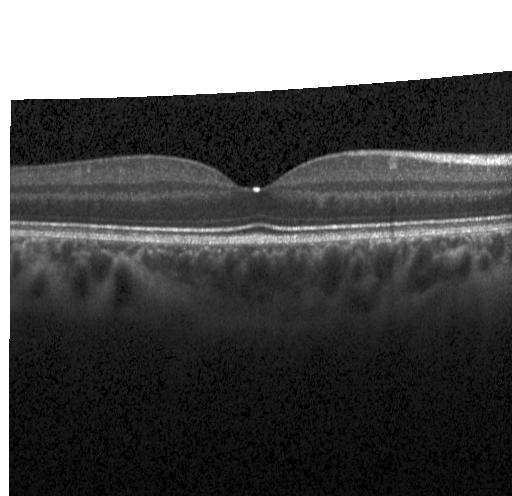

SD-OCT, instrument: Heidelberg Spectralis, retinal OCT B-scan, centered on the fovea. This B-scan demonstrates neither CNV, DME, nor drusen.